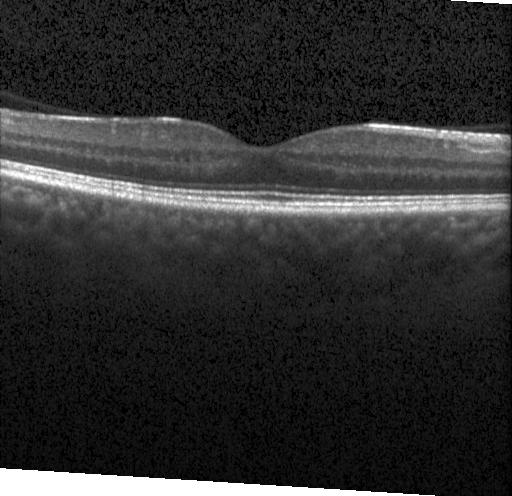 This B-scan demonstrates neither choroidal neovascularization, diabetic macular edema, nor drusen.